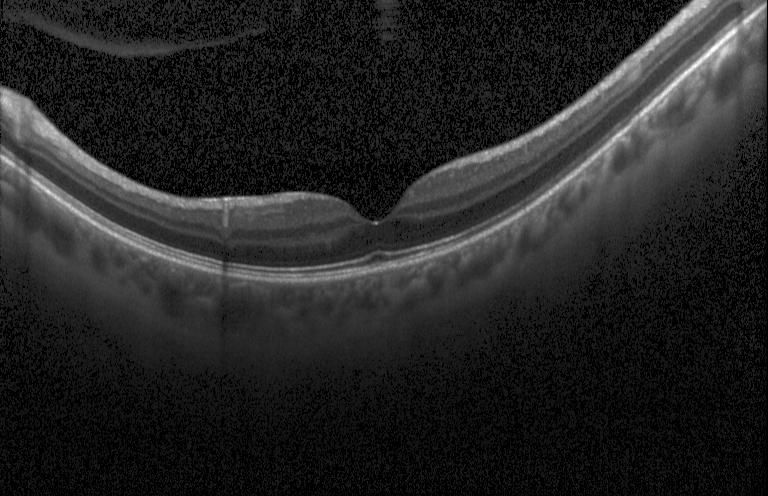 Acquired on a Heidelberg Spectralis. Optical coherence tomography B-scan. Spectral-domain OCT. Through the macula.
OCT finding: no evidence of CNV, DME, or drusen.